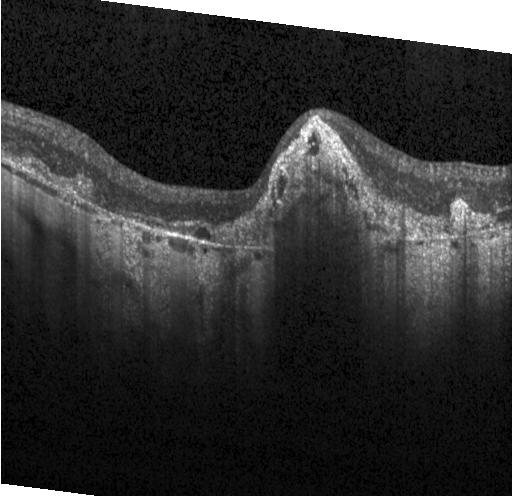 OCT line scan, spectral-domain optical coherence tomography. A choroidal neovascular membrane.